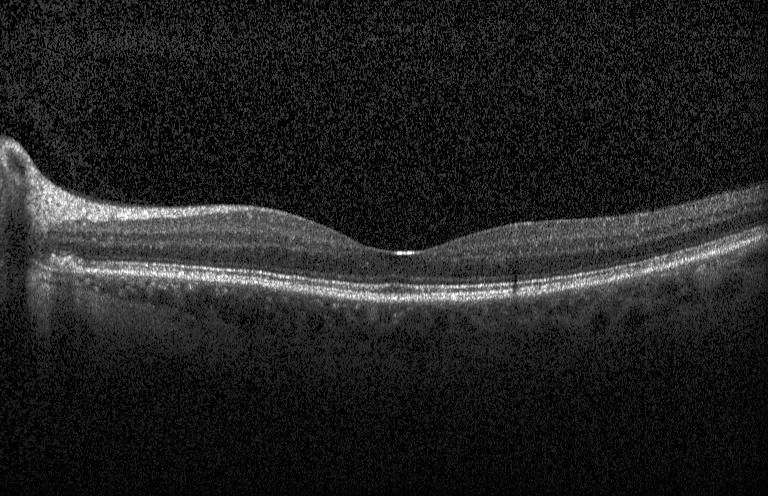

SD-OCT, horizontal scan through the fovea, instrument: Heidelberg Spectralis, OCT line scan
The scan shows neither choroidal neovascularization, diabetic macular edema, nor drusen.